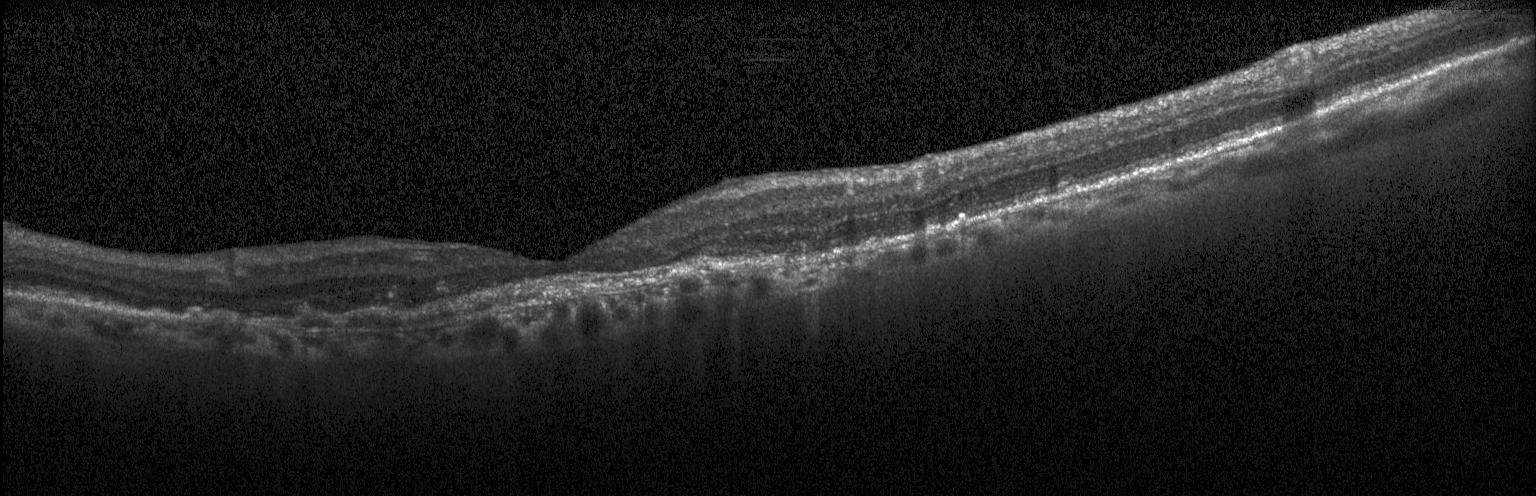

OCT scan showing choroidal neovascularization (CNV).